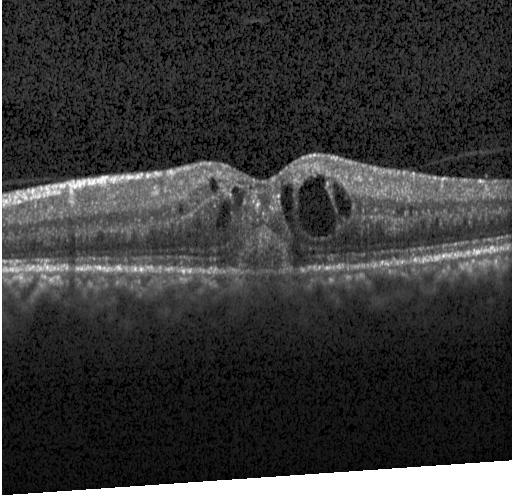

Heidelberg Spectralis OCT system; OCT line scan. Finding: a choroidal neovascular membrane.